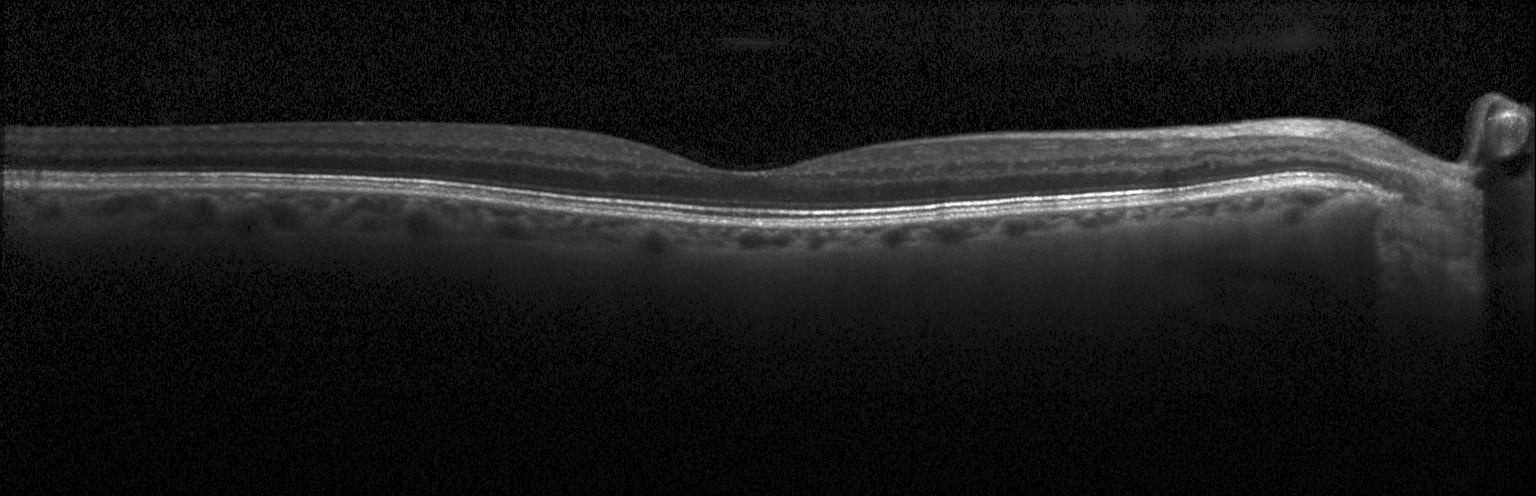 SD-OCT, Heidelberg Spectralis, optical coherence tomography scan.
Dx: no evidence of CNV, DME, or drusen.